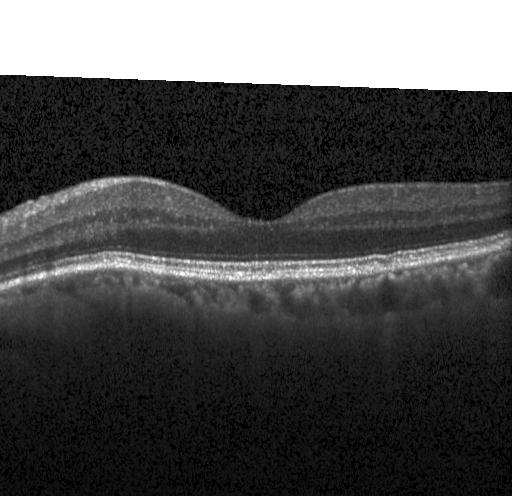 Heidelberg Spectralis OCT system; optical coherence tomography B-scan; SD-OCT — Finding: no choroidal neovascularization, no diabetic macular edema, and no drusen.